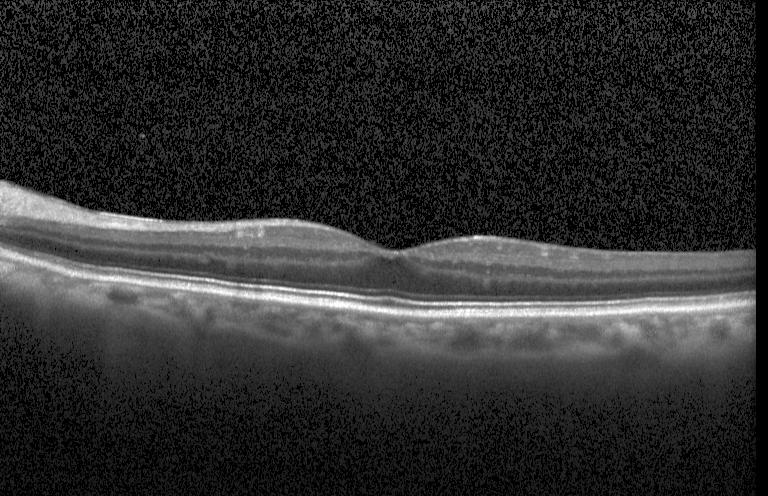
Macular OCT: neither choroidal neovascularization, diabetic macular edema, nor drusen.